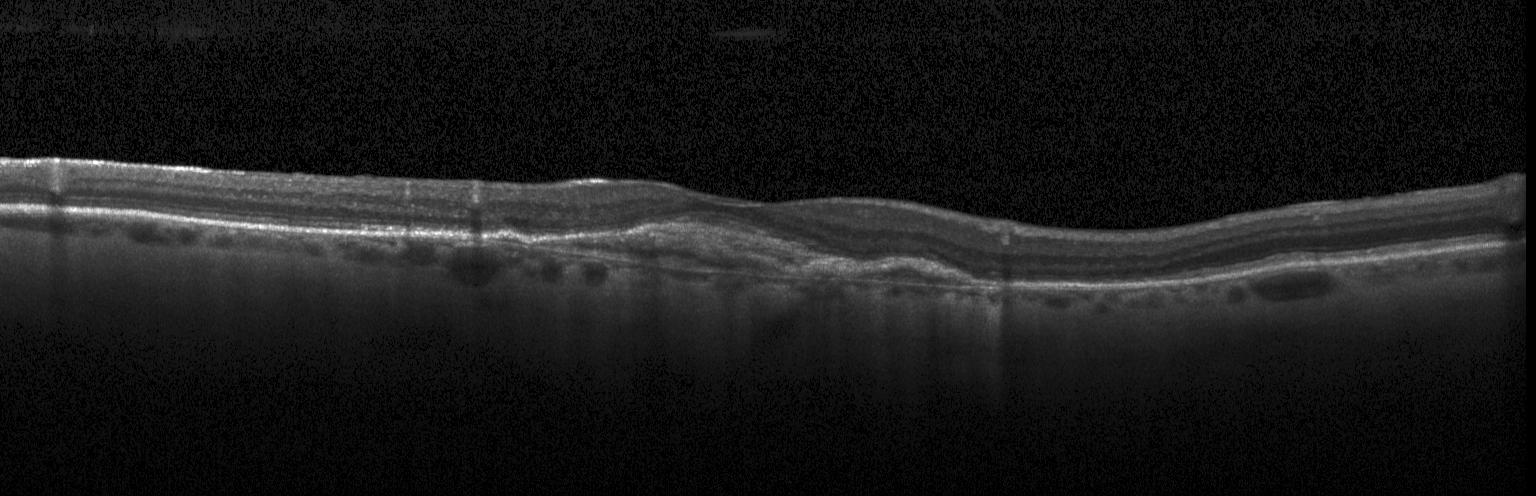
OCT line scan; spectral-domain optical coherence tomography; horizontal scan through the fovea; Heidelberg Spectralis OCT system. Impression: CNV.